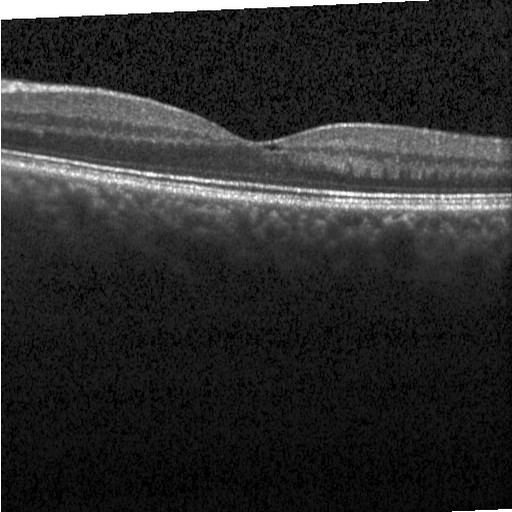

Retinal OCT cross-section, instrument: Heidelberg Spectralis, horizontal scan through the fovea — Dx: DME.